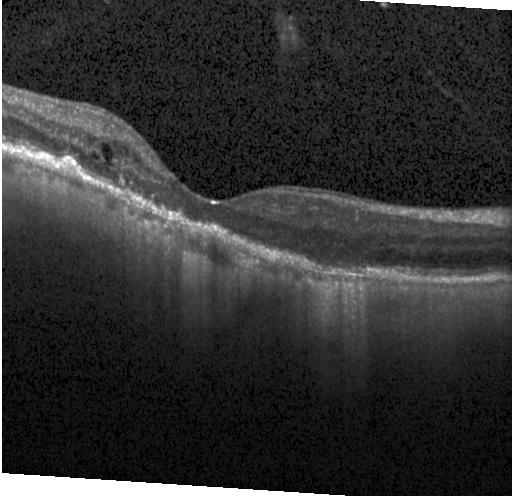
Retinal OCT cross-section. Through the macula. Heidelberg Spectralis. Spectral-domain optical coherence tomography — This B-scan demonstrates a choroidal neovascular membrane.